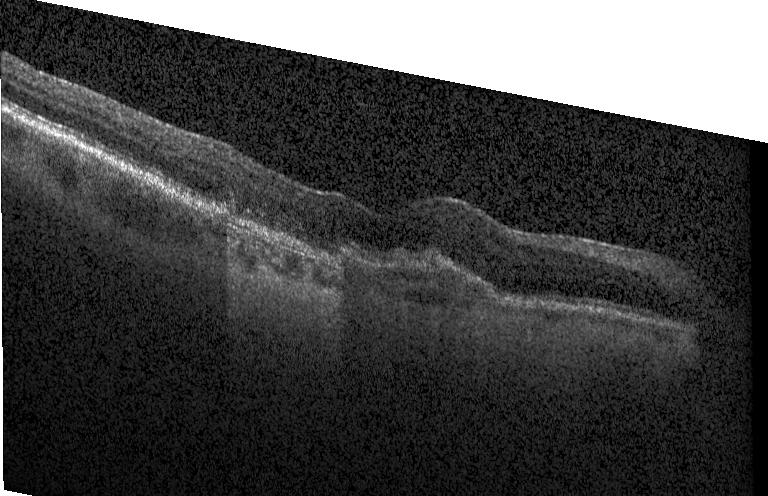
Spectral-domain OCT · optical coherence tomography B-scan · fovea-centered — Impression: a choroidal neovascular membrane.